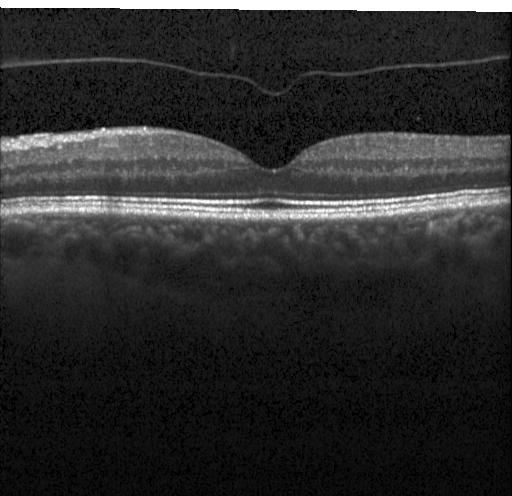

Finding: no choroidal neovascularization, no diabetic macular edema, and no drusen.